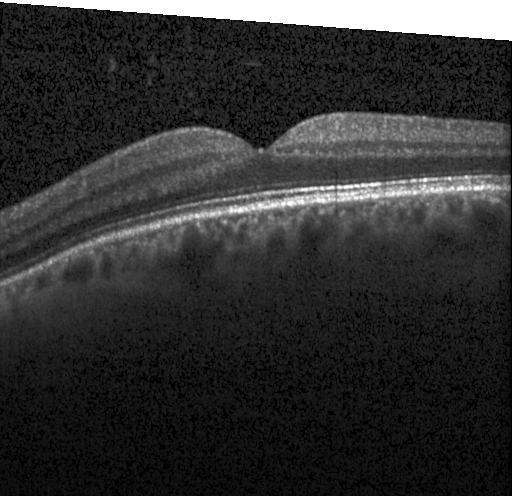
OCT B-scan.
The scan shows no evidence of choroidal neovascularization, diabetic macular edema, or drusen.